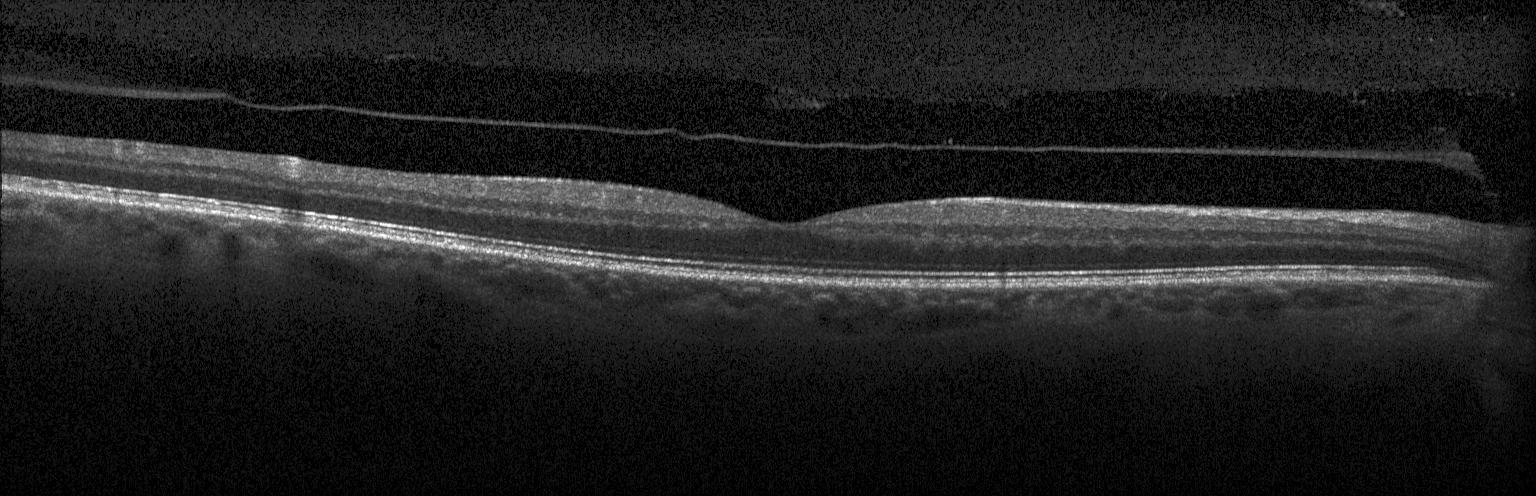

Assessment: no choroidal neovascularization, no diabetic macular edema, and no drusen.